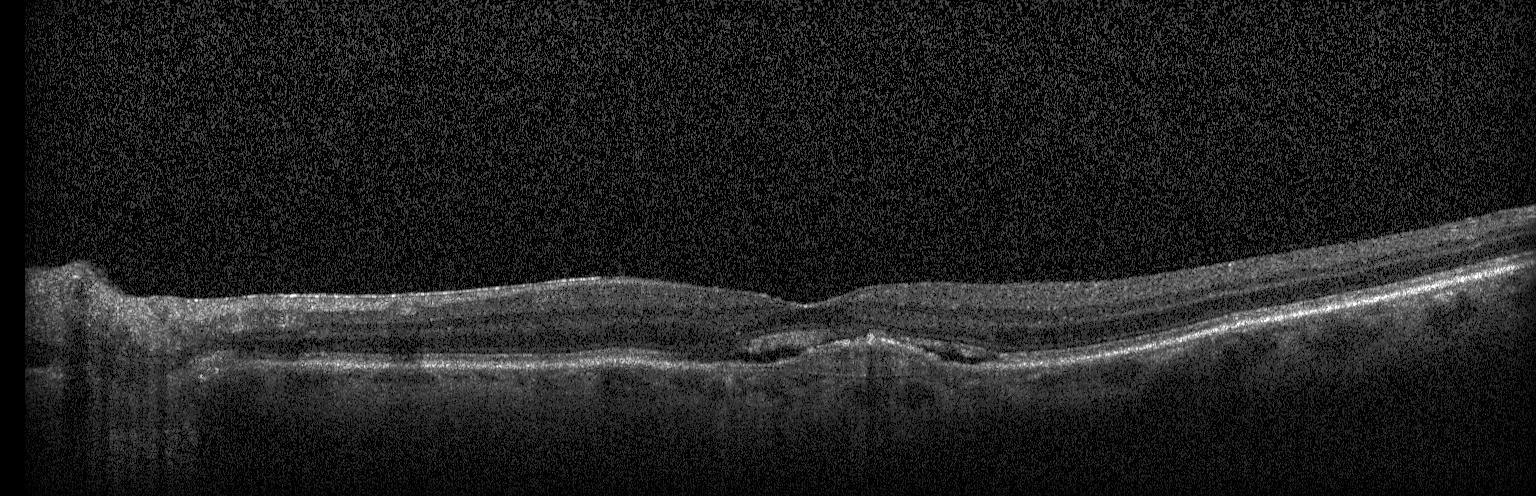
Retinal OCT B-scan · Heidelberg Spectralis — The scan shows a choroidal neovascular membrane.